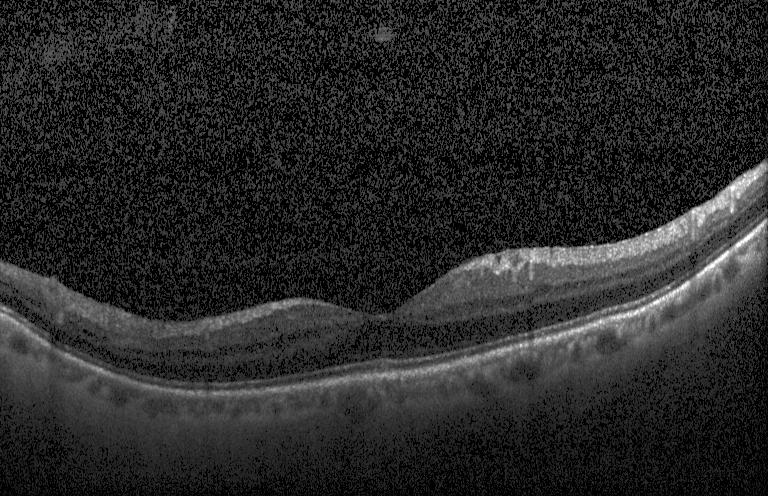 Heidelberg Spectralis; through the macula; OCT B-scan; spectral-domain OCT — Impression: neither choroidal neovascularization, diabetic macular edema, nor drusen.